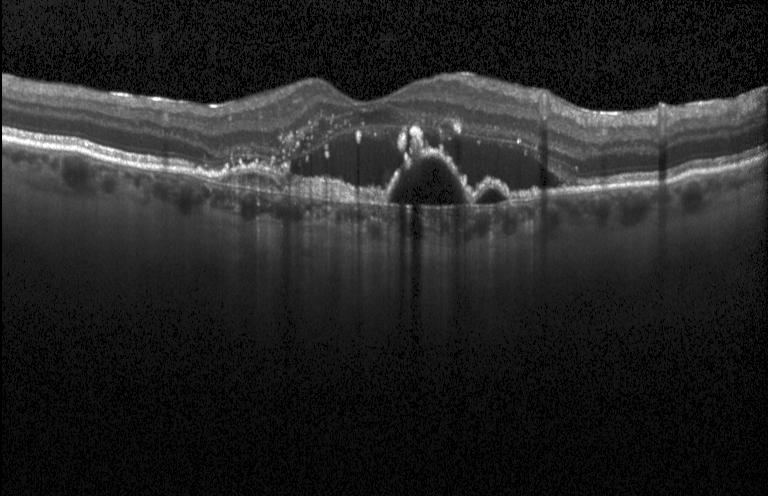

Assessment: CNV.